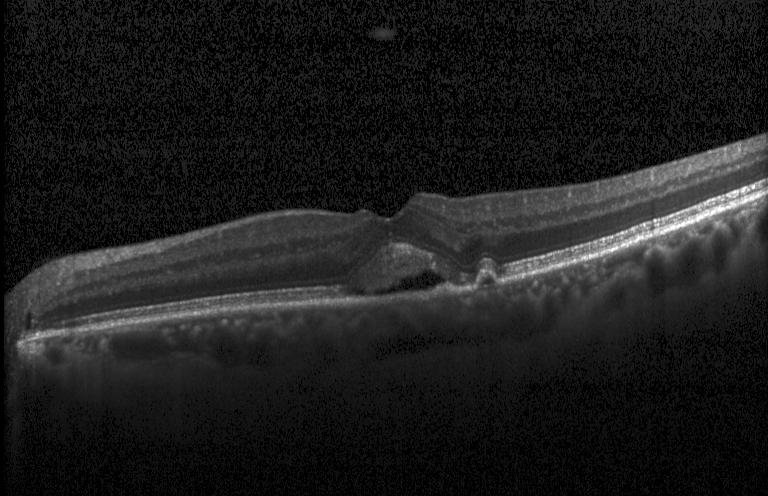 Dx: a choroidal neovascular membrane.